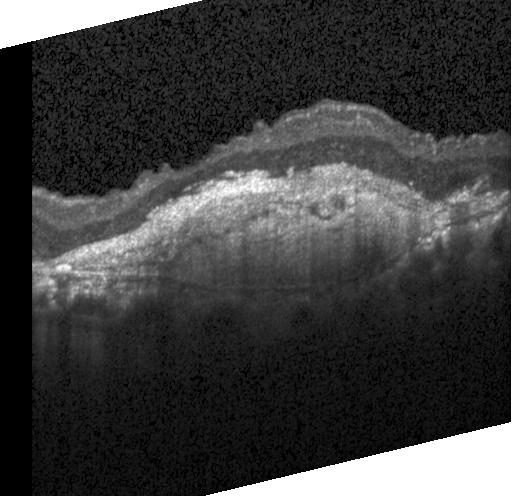

SD-OCT, centered on the fovea, retinal OCT B-scan.
Finding: choroidal neovascularization (CNV).